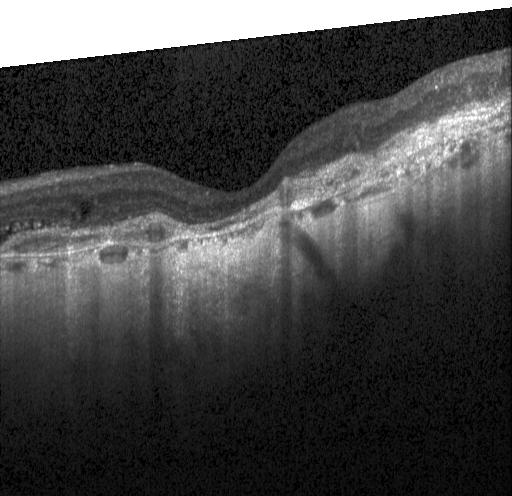 OCT B-scan showing choroidal neovascularization (CNV).